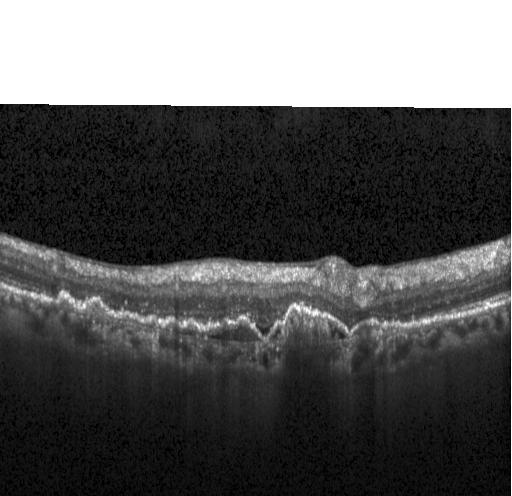
Finding: a choroidal neovascular membrane.